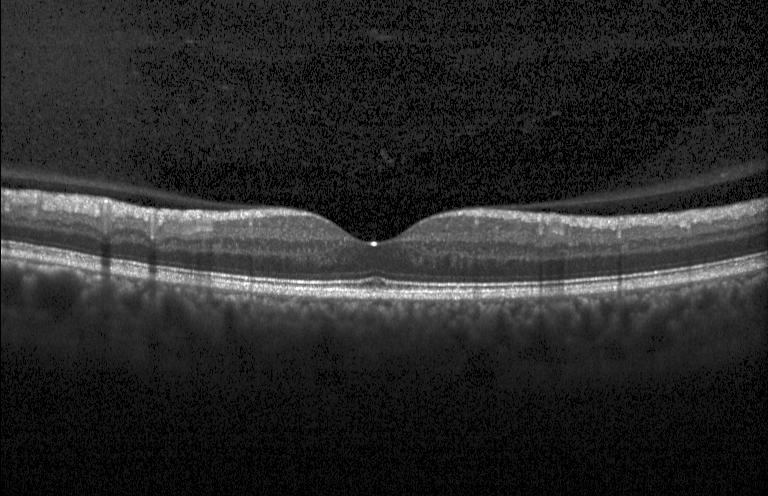 OCT B-scan showing no evidence of CNV, DME, or drusen.